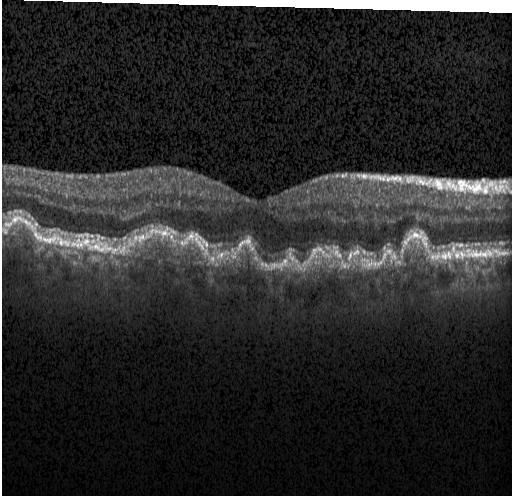 OCT finding: sub-RPE drusenoid deposits.